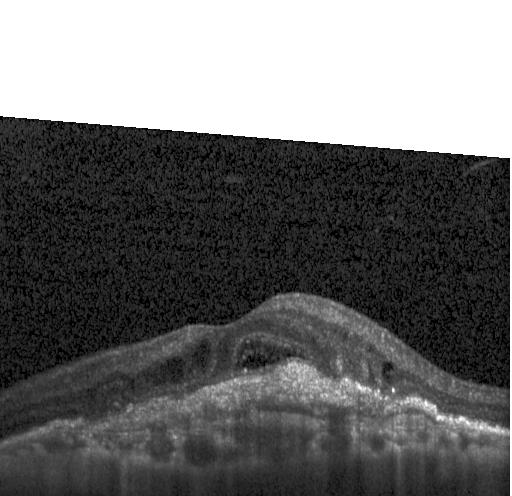
Assessment: a choroidal neovascular membrane.